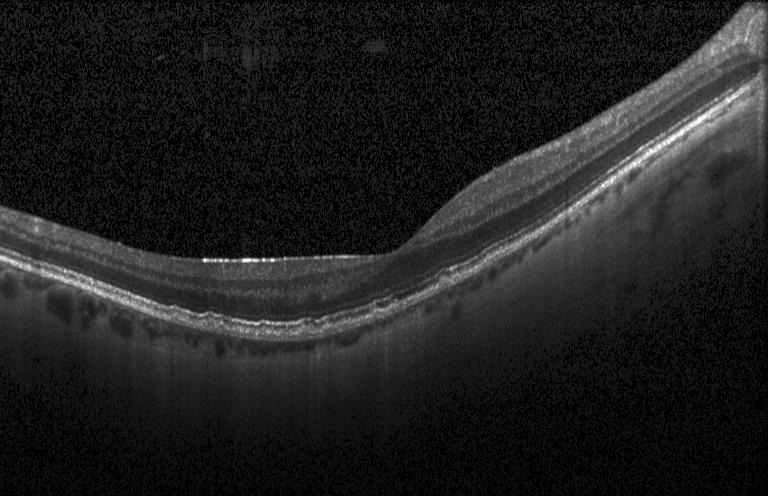
OCT B-scan showing drusen.